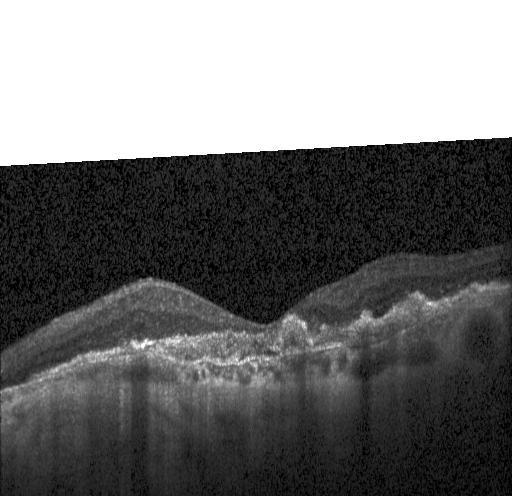

Retinal OCT cross-section showing a choroidal neovascular membrane.